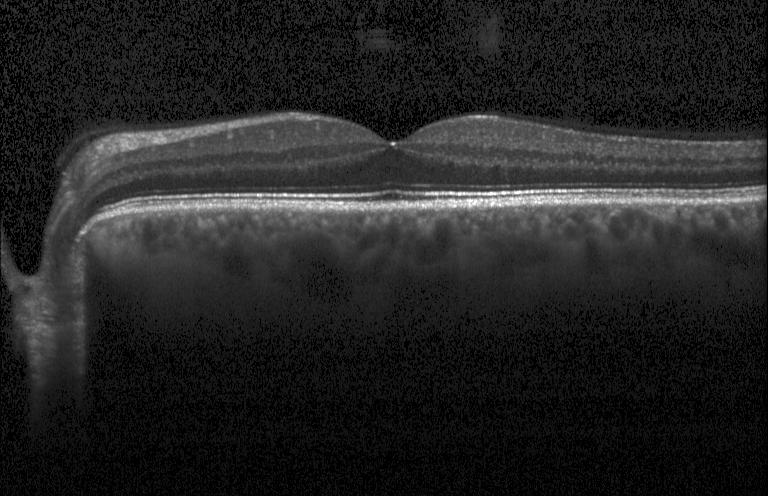 OCT line scan; acquired on a Heidelberg Spectralis; SD-OCT.
This B-scan demonstrates no choroidal neovascularization, no diabetic macular edema, and no drusen.